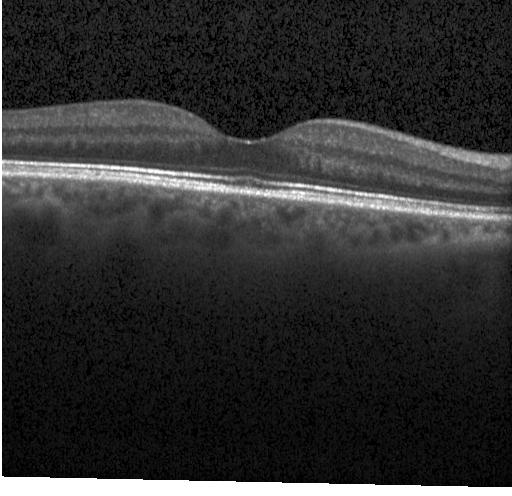

Acquired on a Heidelberg Spectralis; spectral-domain OCT; retinal OCT B-scan
No choroidal neovascularization, no diabetic macular edema, and no drusen.